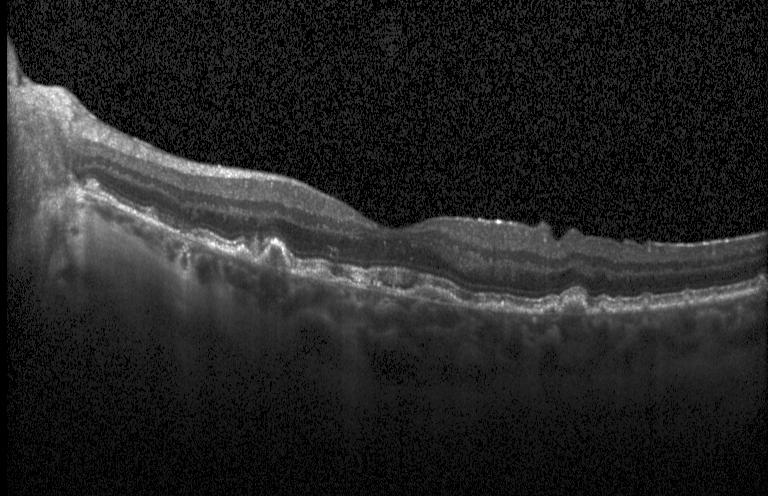 Spectral-domain optical coherence tomography, through the macula, OCT B-scan.
This B-scan demonstrates choroidal neovascularization (CNV).